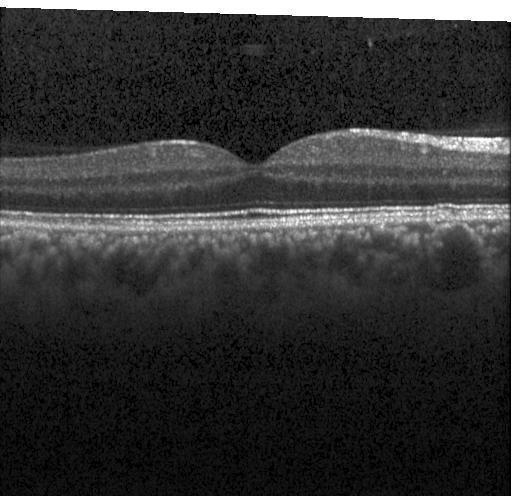 Optical coherence tomography scan — This B-scan demonstrates no evidence of CNV, DME, or drusen.